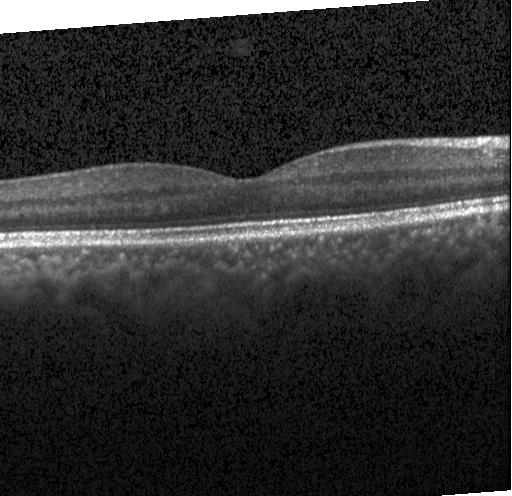 No evidence of choroidal neovascularization, diabetic macular edema, or drusen.